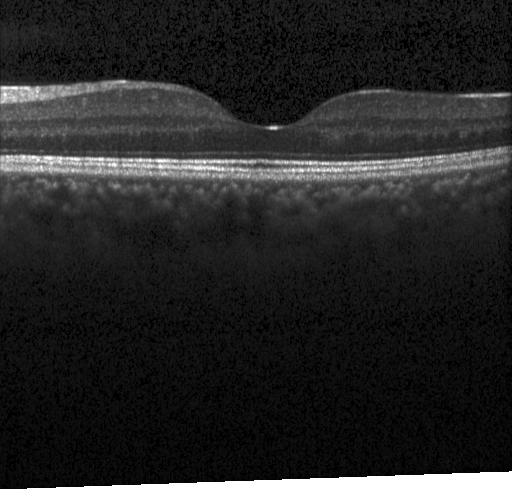

OCT line scan
This B-scan demonstrates no choroidal neovascularization, no diabetic macular edema, and no drusen.